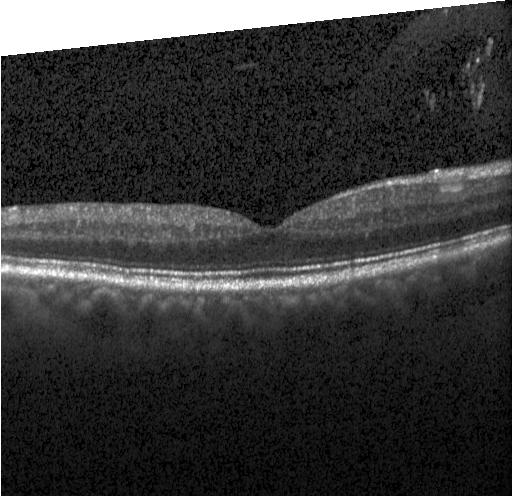 Spectral-domain OCT B-scan: neither choroidal neovascularization, diabetic macular edema, nor drusen.